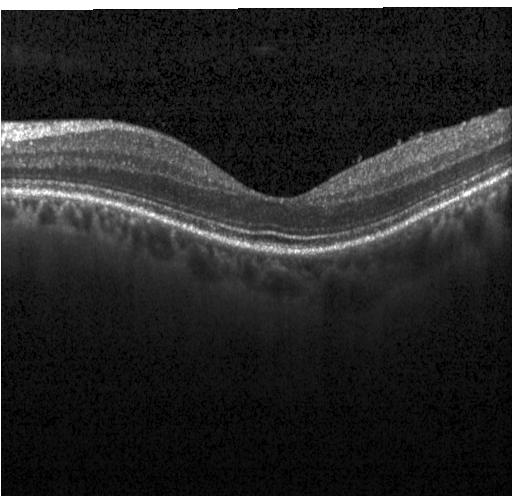

Spectral-domain optical coherence tomography; optical coherence tomography scan; through the macula
OCT finding: no choroidal neovascularization, no diabetic macular edema, and no drusen.